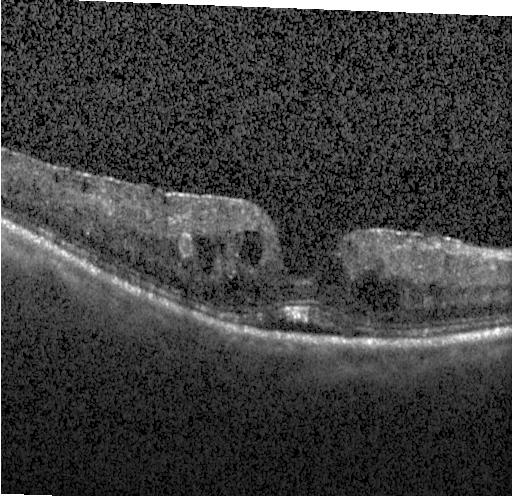 Dx: diabetic macular edema.